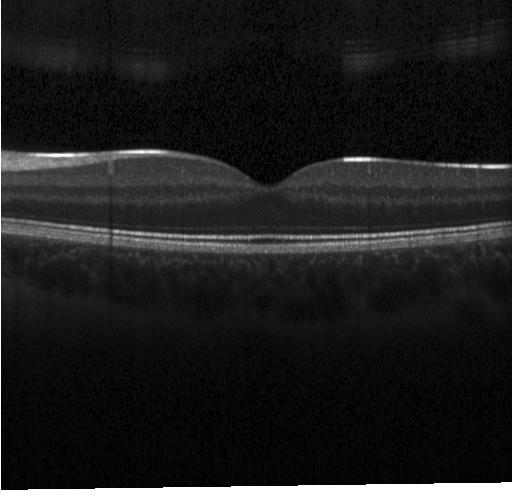

No evidence of choroidal neovascularization, diabetic macular edema, or drusen.